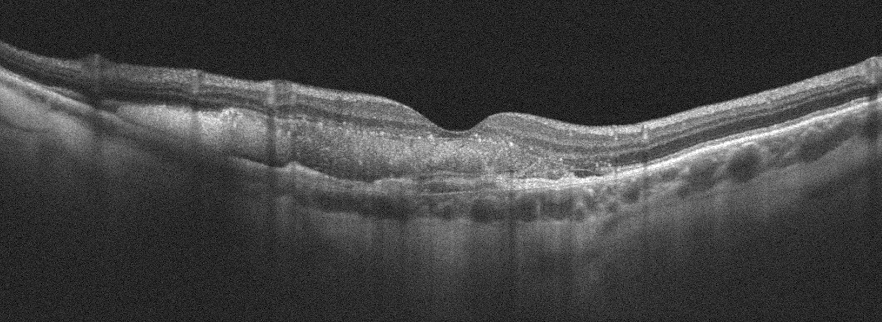 Left eye, retinal OCT B-scan — Assessment: age-related macular degeneration.